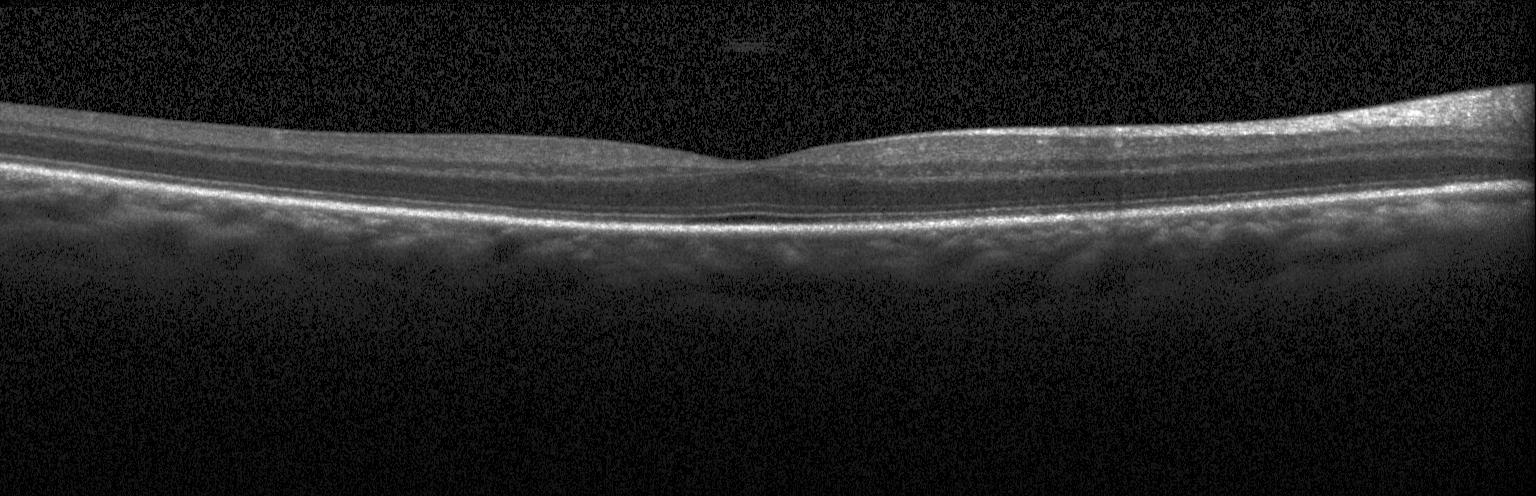

Retinal OCT cross-section showing neither choroidal neovascularization, diabetic macular edema, nor drusen.